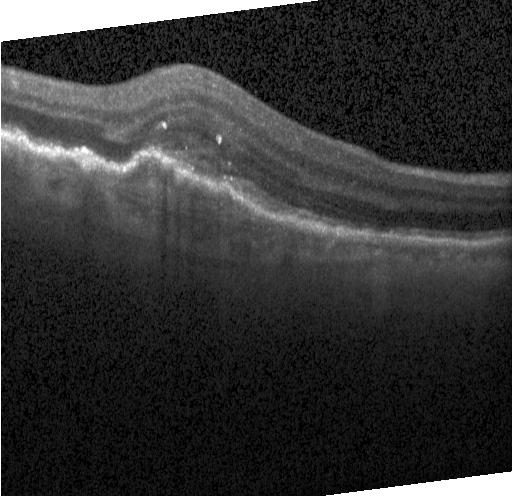 Diagnosis: a choroidal neovascular membrane.